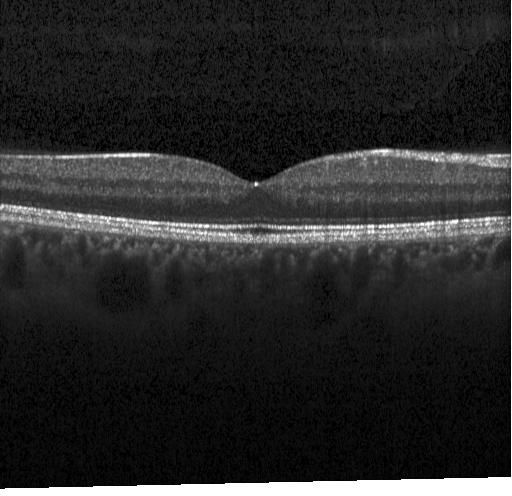

Assessment: neither choroidal neovascularization, diabetic macular edema, nor drusen.